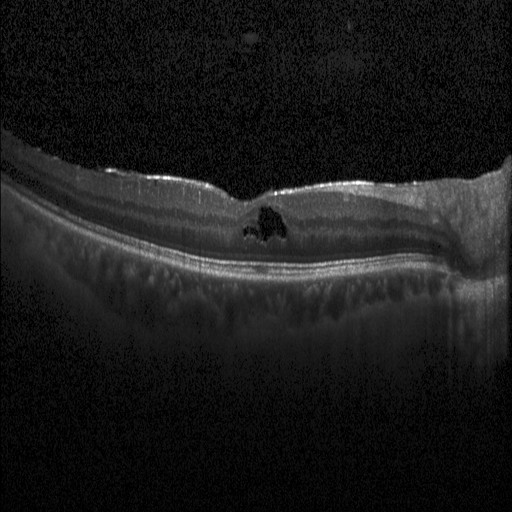
The scan shows diabetic macular edema.